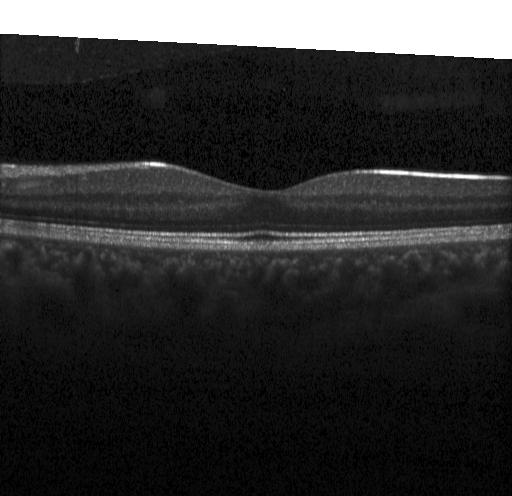

OCT scan showing no choroidal neovascularization, no diabetic macular edema, and no drusen.